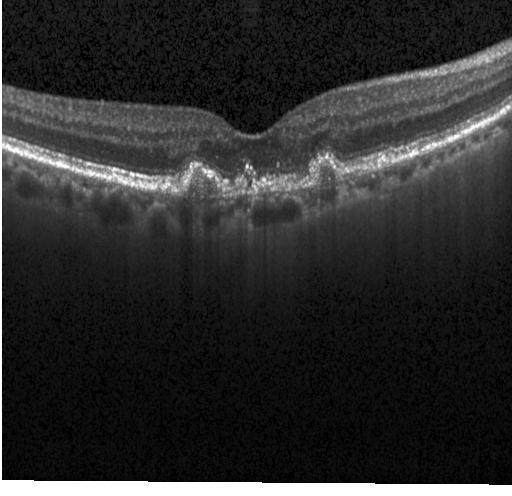

OCT B-scan showing sub-RPE drusenoid deposits.